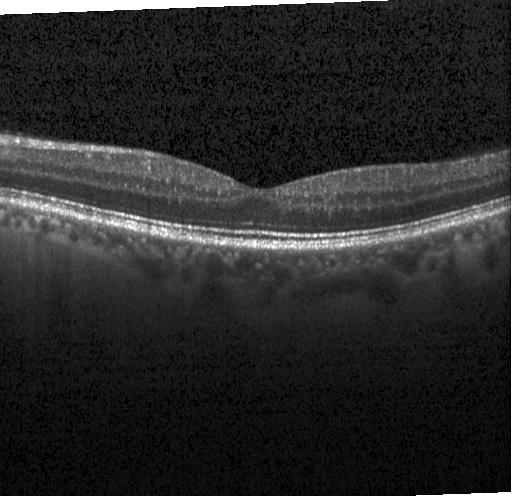 Through the macula · OCT B-scan — Impression: no CNV, no DME, and no drusen.